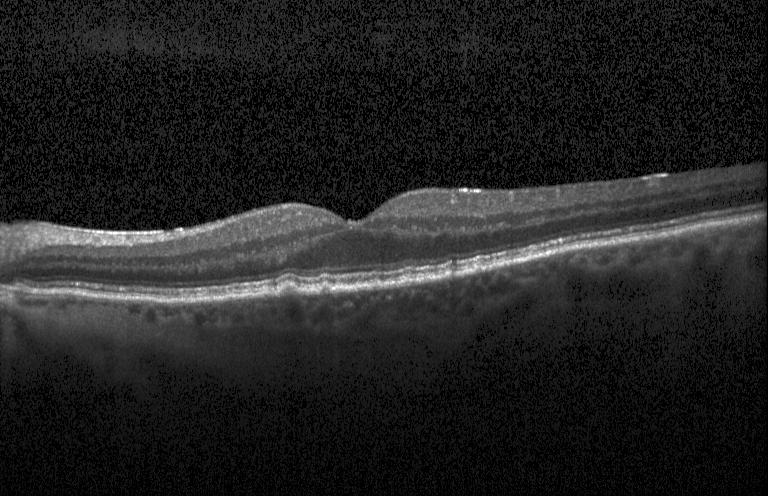
Macular scan, optical coherence tomography scan, instrument: Heidelberg Spectralis.
This B-scan demonstrates drusen.